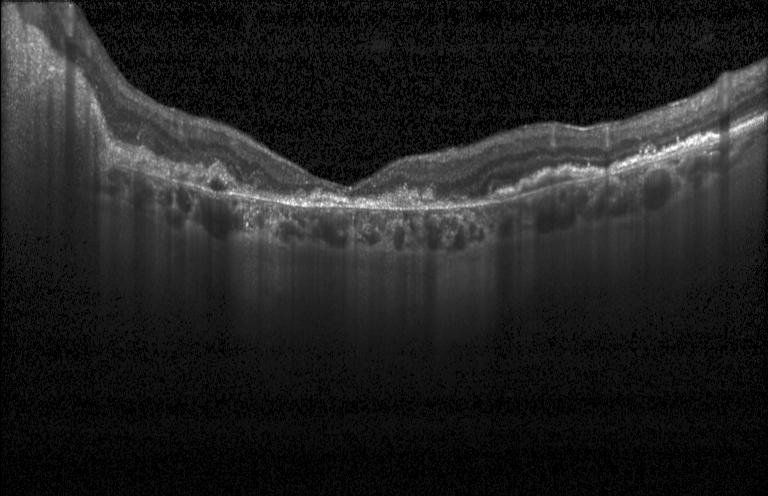
Heidelberg Spectralis. Retinal OCT cross-section. Macular scan.
Dx: a choroidal neovascular membrane.